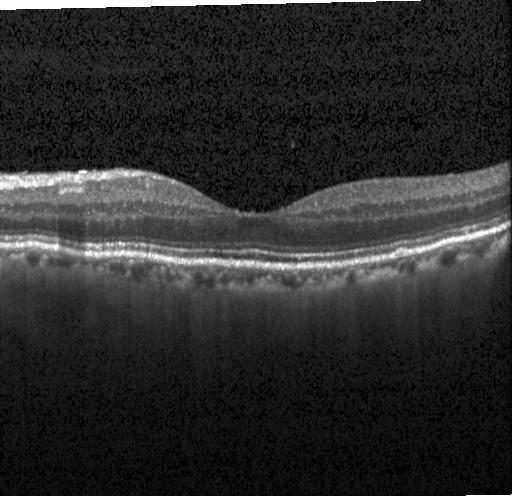

Optical coherence tomography scan. Impression: neither choroidal neovascularization, diabetic macular edema, nor drusen.